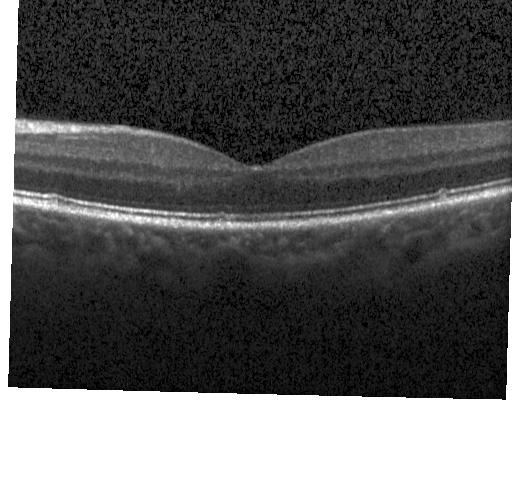 OCT finding: drusen.